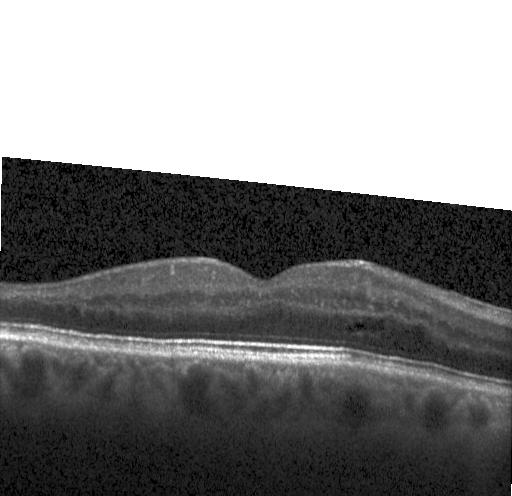
This B-scan demonstrates DME.